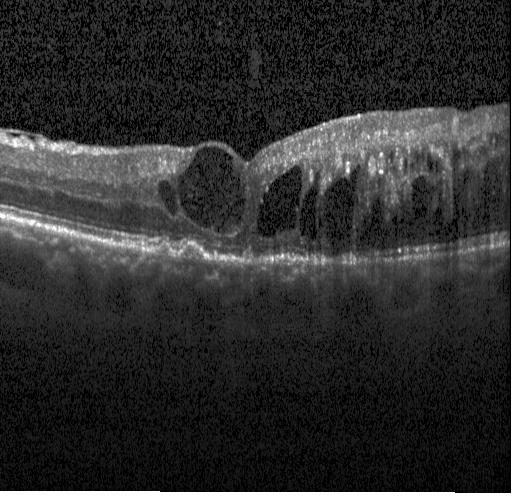 OCT line scan.
OCT finding: diabetic macular edema (DME).